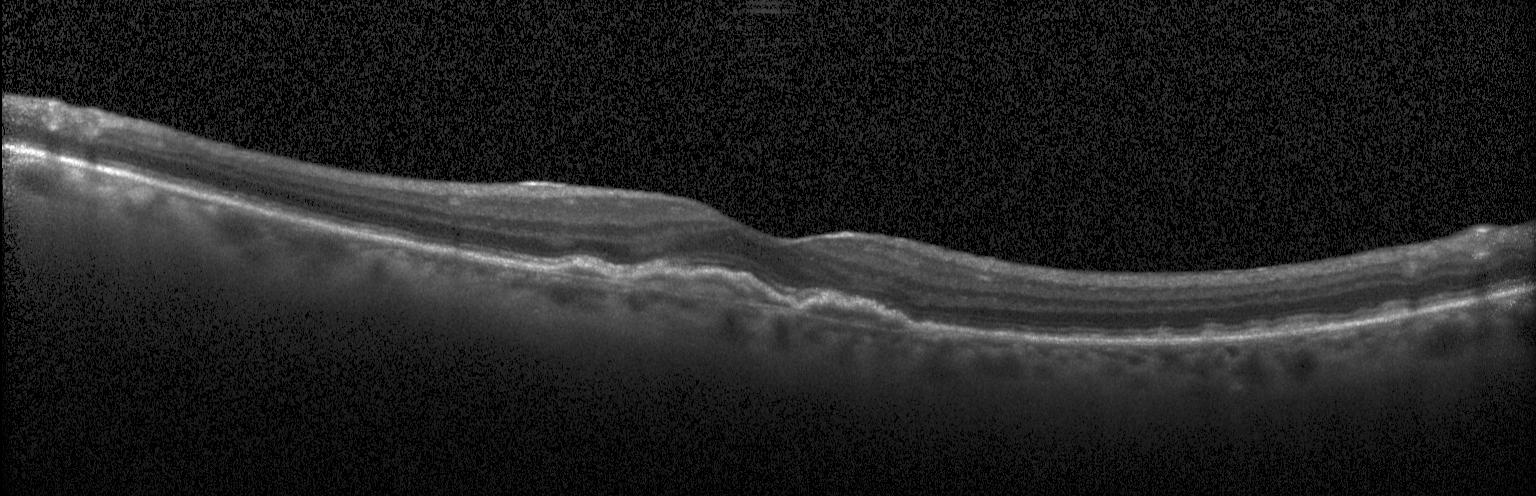 Retinal OCT cross-section
OCT finding: a choroidal neovascular membrane.